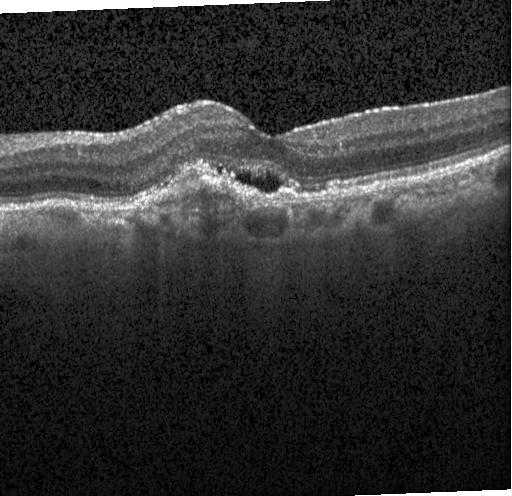

OCT scan showing choroidal neovascularization (CNV).